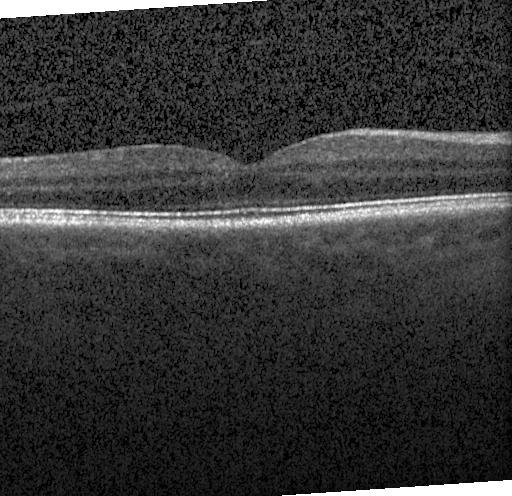

Acquired on a Heidelberg Spectralis. Optical coherence tomography scan.
OCT finding: no choroidal neovascularization, no diabetic macular edema, and no drusen.